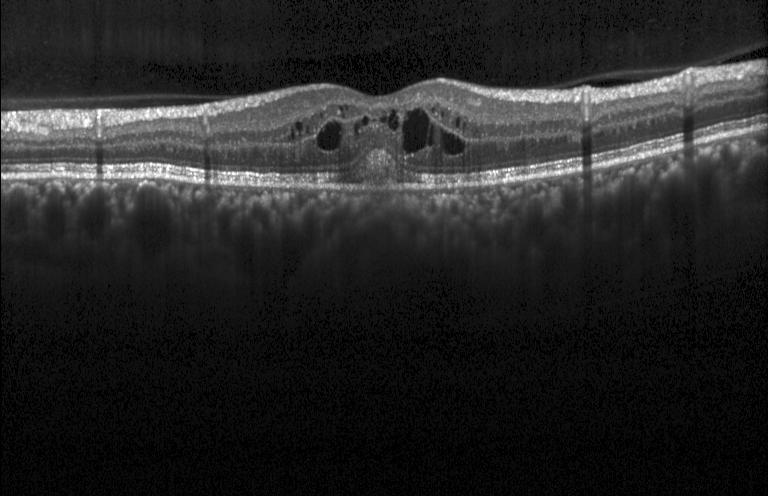 Spectral-domain OCT B-scan: CNV.